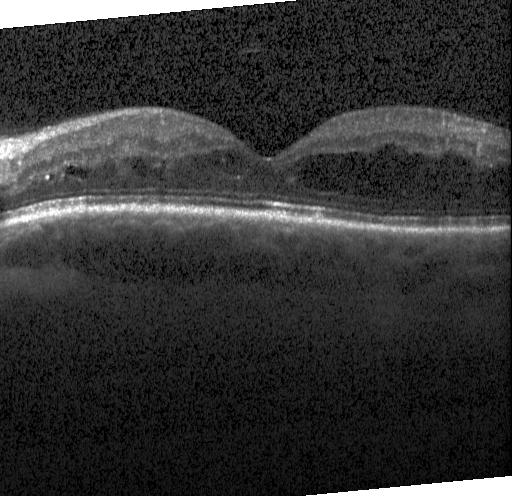

Retinal OCT B-scan, fovea-centered. DME.